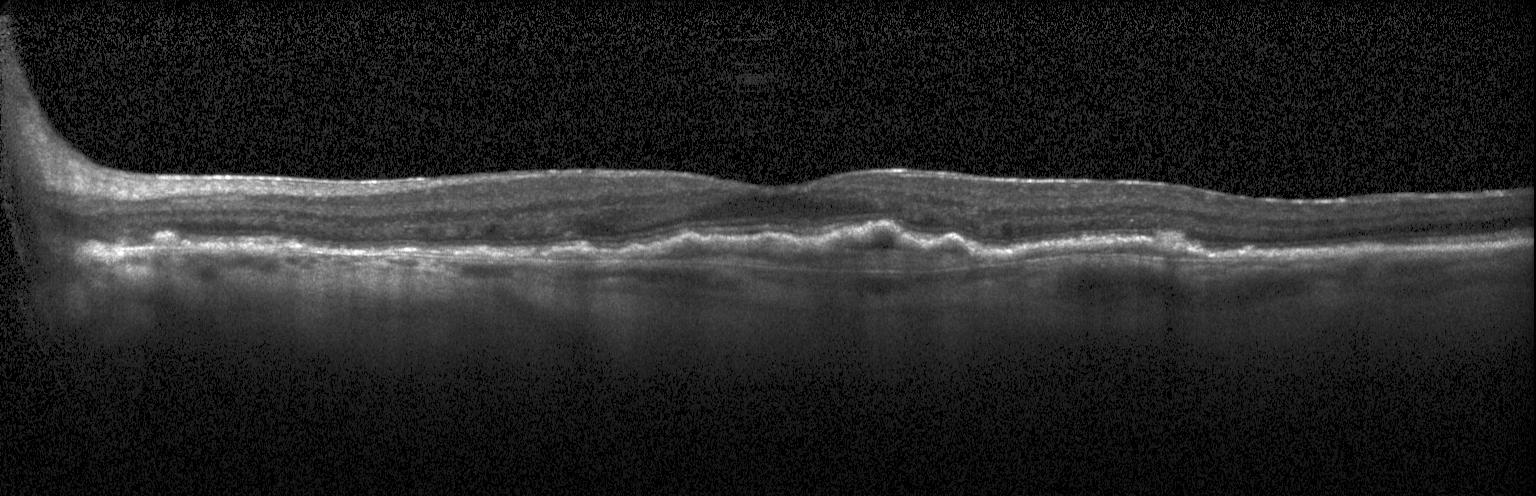 Spectral-domain OCT B-scan: choroidal neovascularization.